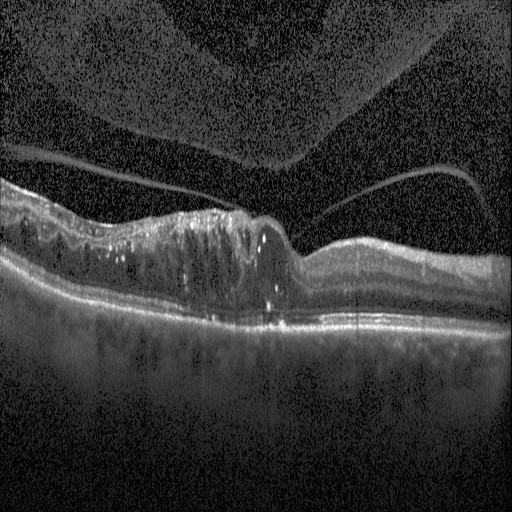
Diagnosis: diabetic macular edema.